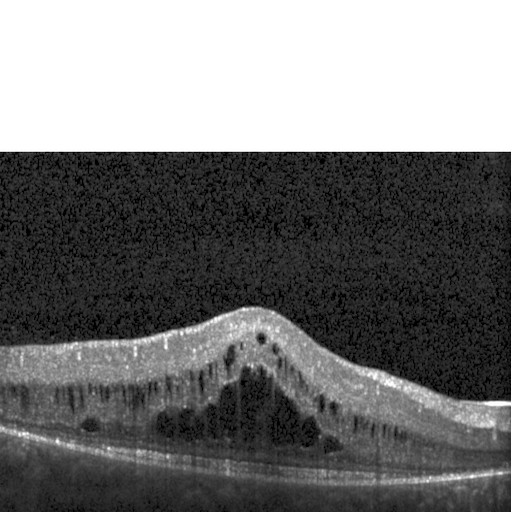
Retinal OCT cross-section; instrument: Heidelberg Spectralis.
Finding: diabetic macular edema.